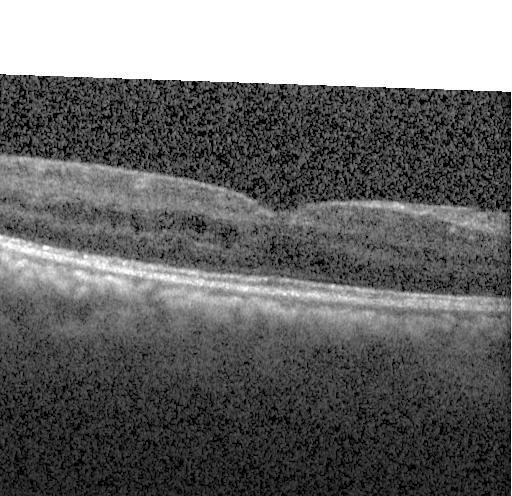
OCT B-scan · through the macula — Macular OCT: diabetic macular edema.